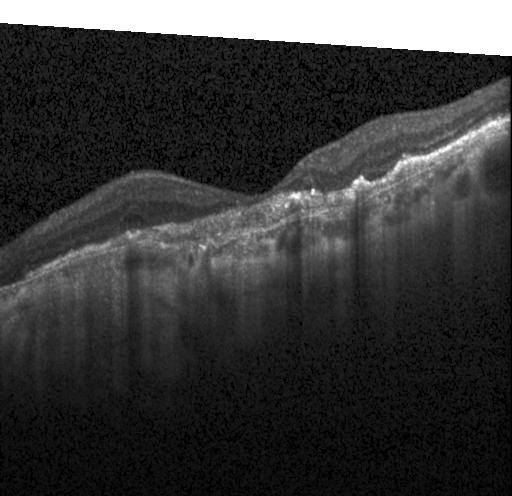
Spectral-domain optical coherence tomography. Macular scan. Retinal OCT B-scan.
Impression: CNV.